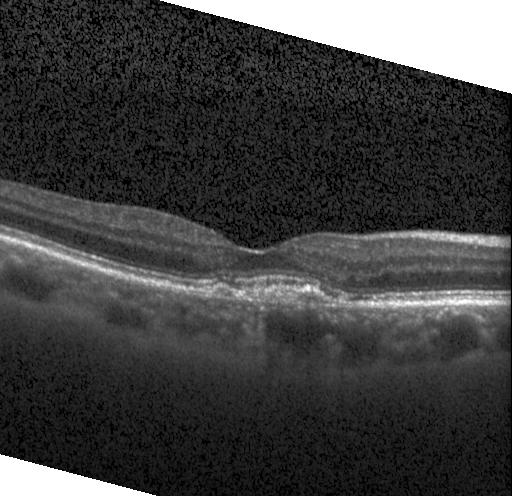

Macular OCT demonstrating CNV.